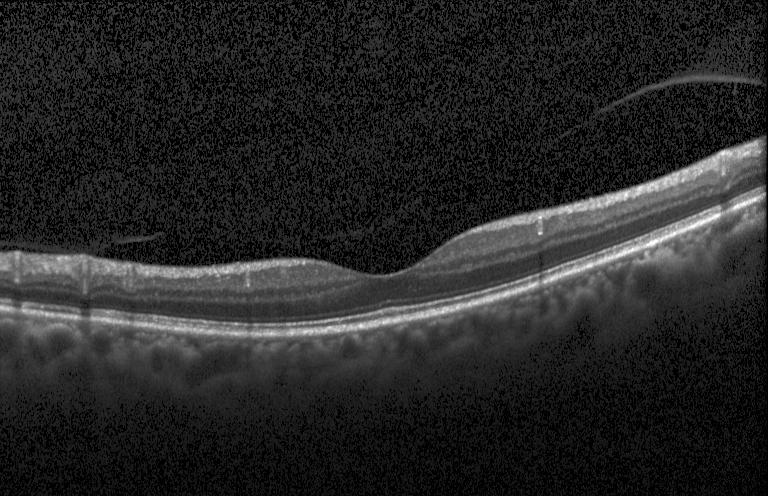
Acquired on a Heidelberg Spectralis, centered on the fovea, OCT B-scan — Impression: neither choroidal neovascularization, diabetic macular edema, nor drusen.